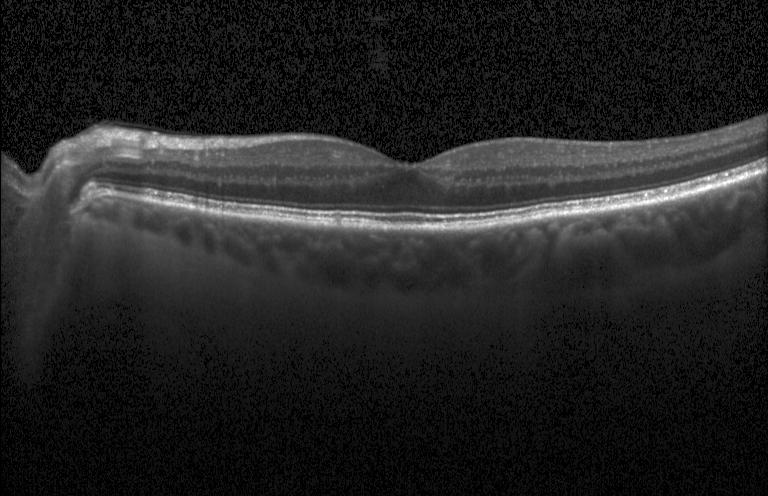
Retinal OCT B-scan. Fovea-centered. Spectral-domain OCT. Heidelberg Spectralis OCT system
Dx: no choroidal neovascularization, no diabetic macular edema, and no drusen.